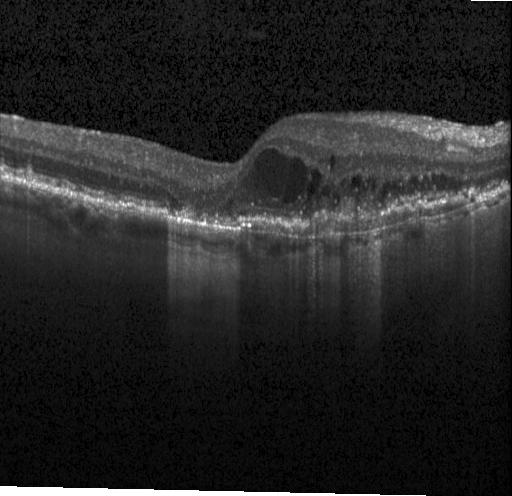
OCT B-scan showing a choroidal neovascular membrane.